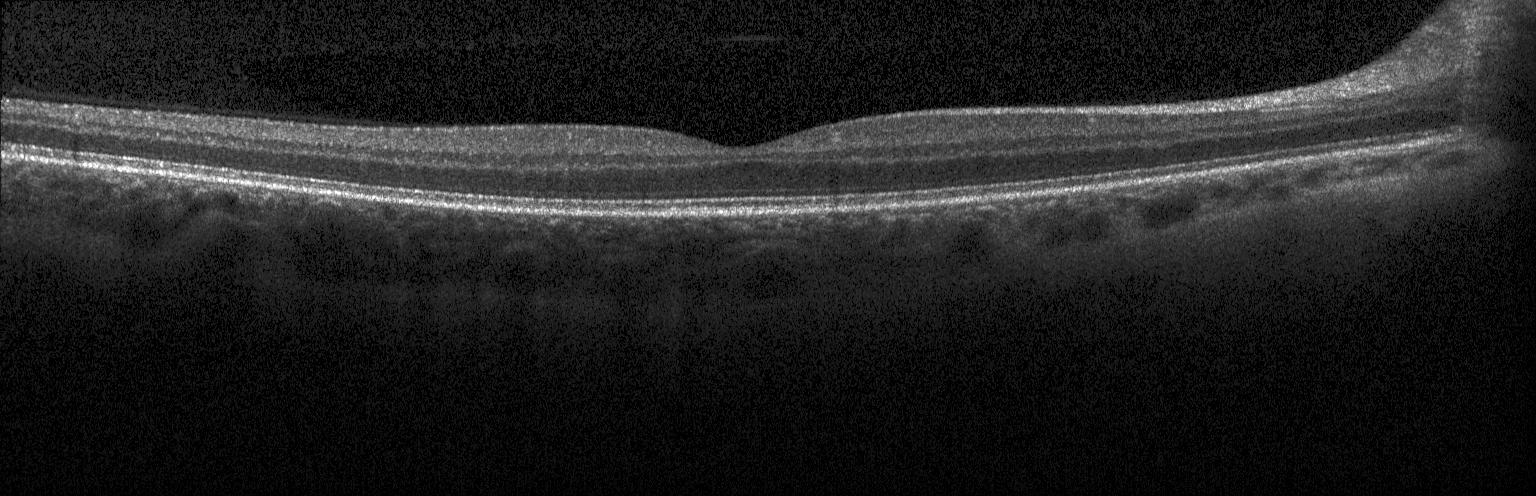
Heidelberg Spectralis, optical coherence tomography B-scan — Diagnosis: no CNV, no DME, and no drusen.